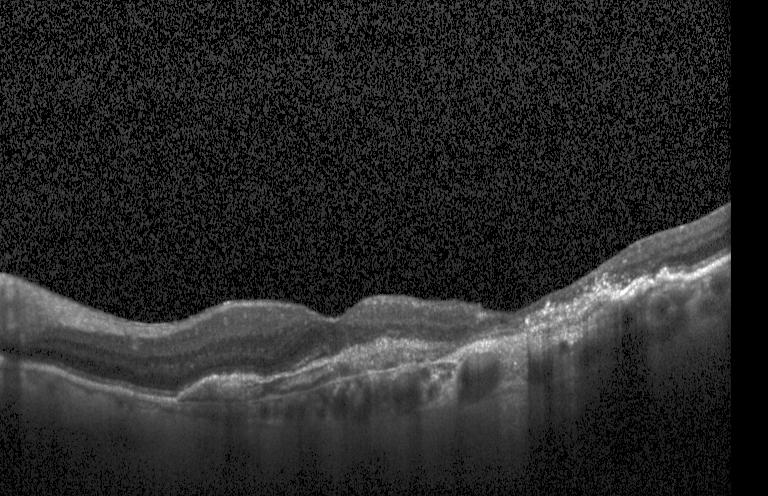

Acquired on a Heidelberg Spectralis · optical coherence tomography scan.
Assessment: CNV.